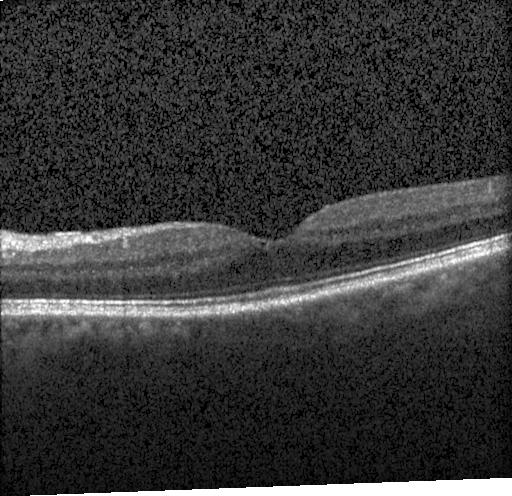

Instrument: Heidelberg Spectralis · spectral-domain optical coherence tomography · optical coherence tomography scan · macular scan.
Diagnosis: no choroidal neovascularization, no diabetic macular edema, and no drusen.